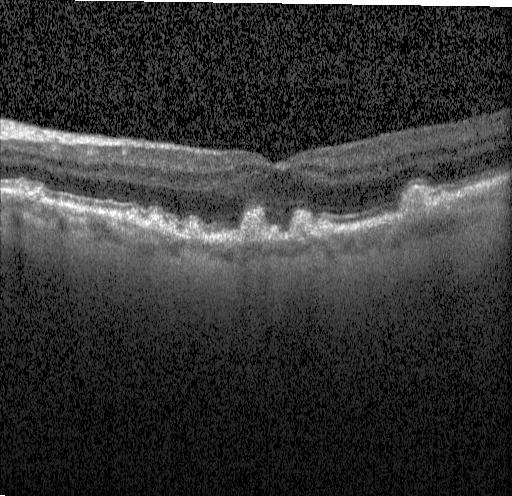

Assessment: multiple drusen.